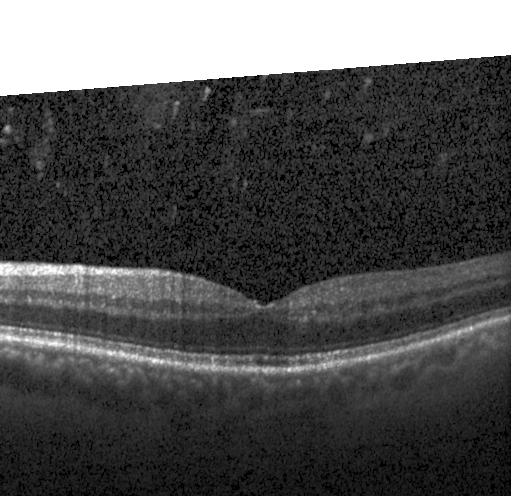
Retinal OCT B-scan. Dx: neither choroidal neovascularization, diabetic macular edema, nor drusen.